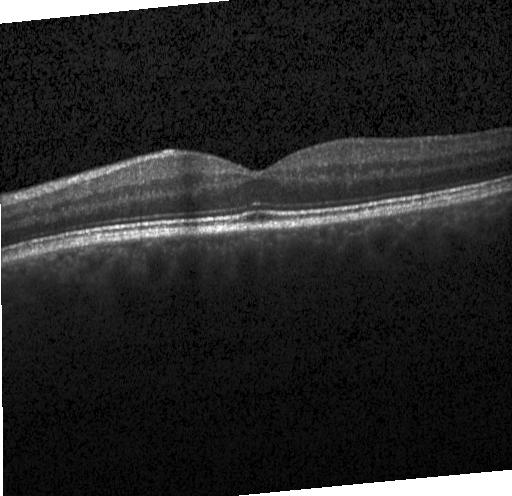
Impression: neither CNV, DME, nor drusen.